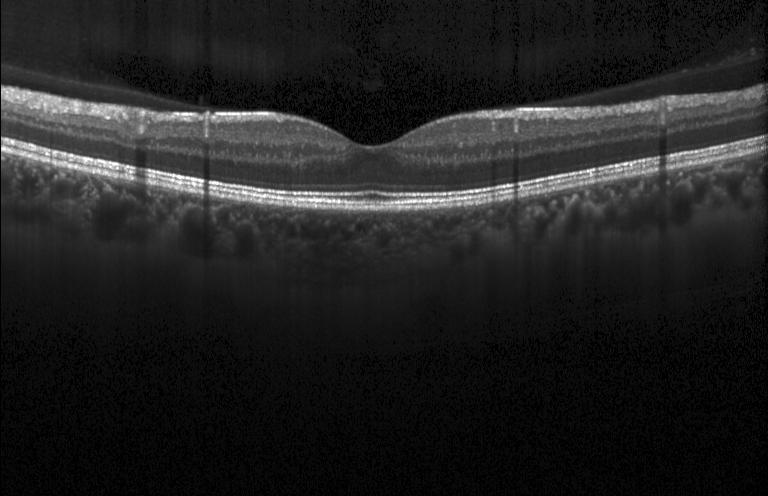 Horizontal scan through the fovea; SD-OCT; OCT B-scan; acquired on a Heidelberg Spectralis — Assessment: neither CNV, DME, nor drusen.